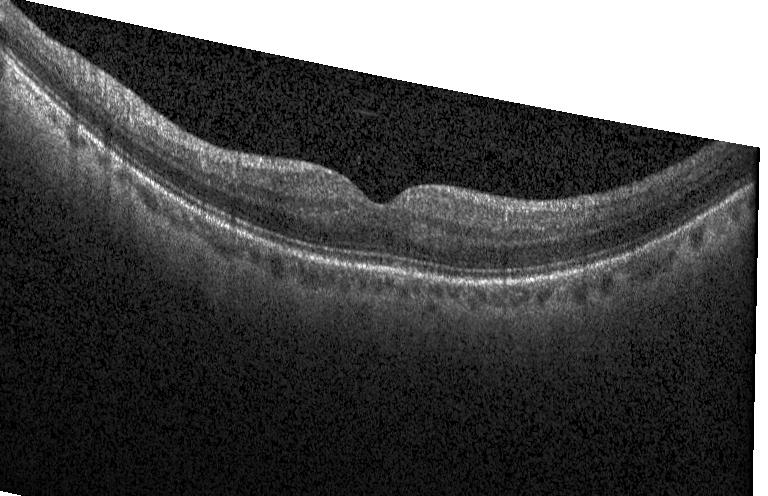

OCT scan showing no choroidal neovascularization, diabetic macular edema, or drusen.